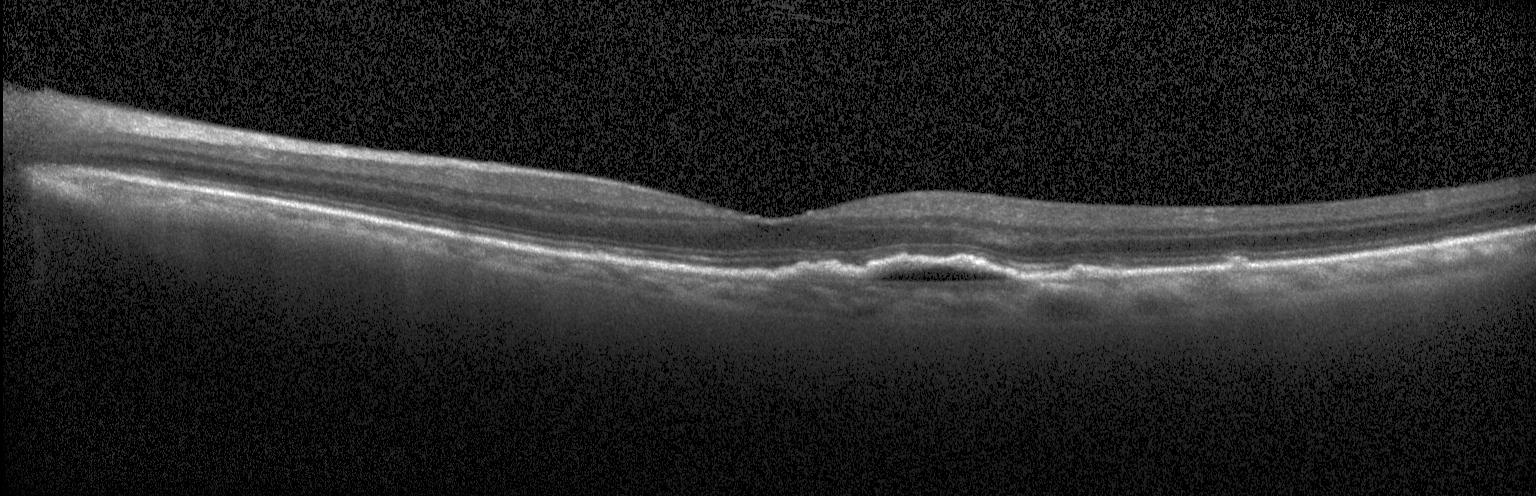 OCT B-scan
Diagnosis: choroidal neovascularization.